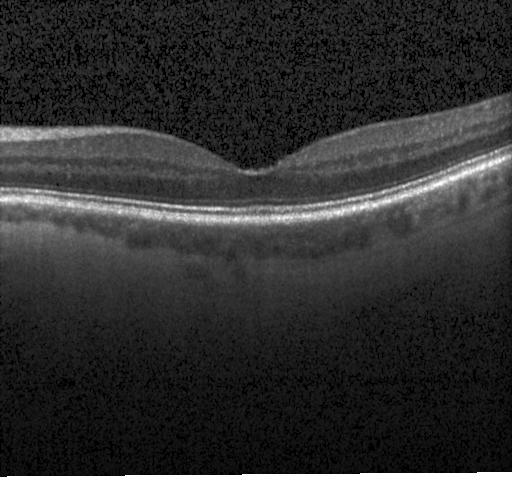
Macular OCT demonstrating neither choroidal neovascularization, diabetic macular edema, nor drusen.